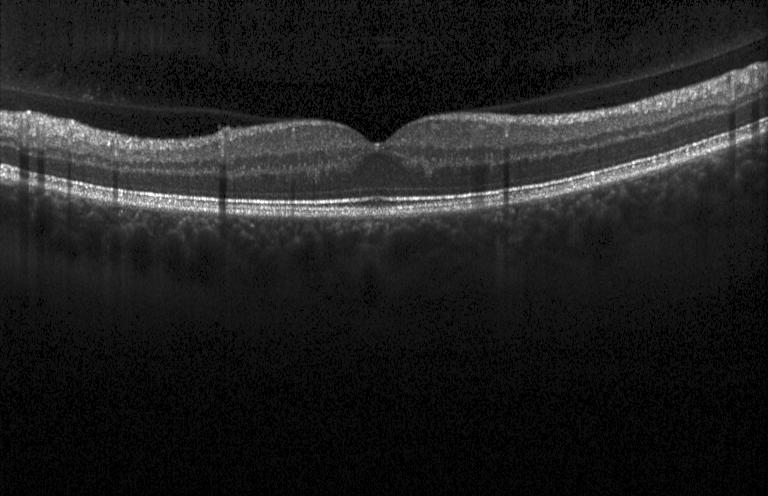 Centered on the fovea; OCT B-scan; spectral-domain OCT; Heidelberg Spectralis OCT system — OCT finding: neither CNV, DME, nor drusen.